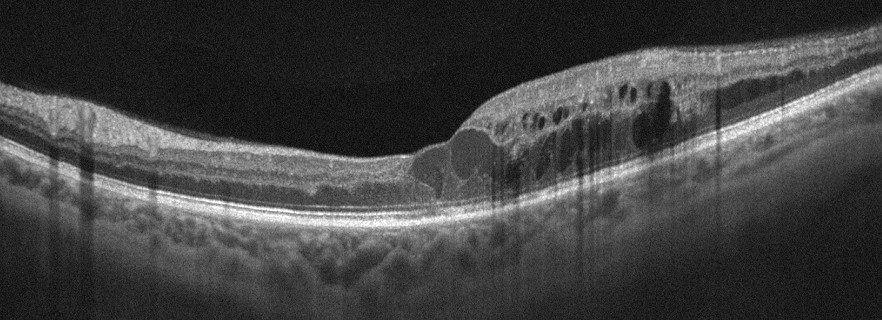 Optical coherence tomography B-scan. Finding: diabetic macular edema (DME).